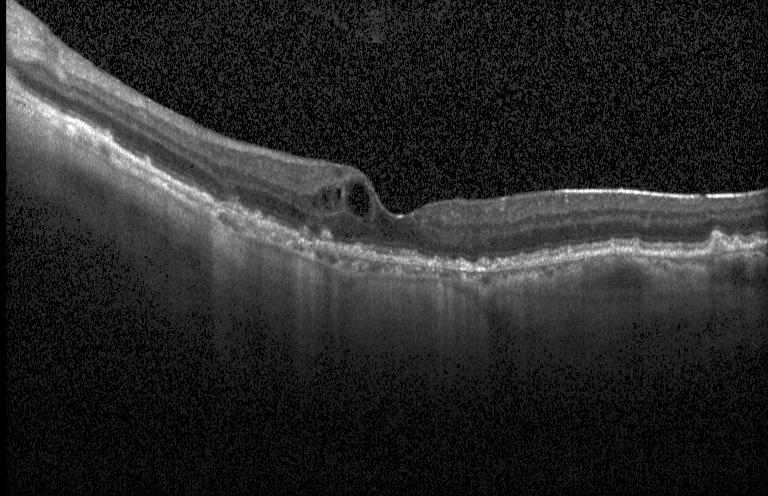
OCT finding: a choroidal neovascular membrane.